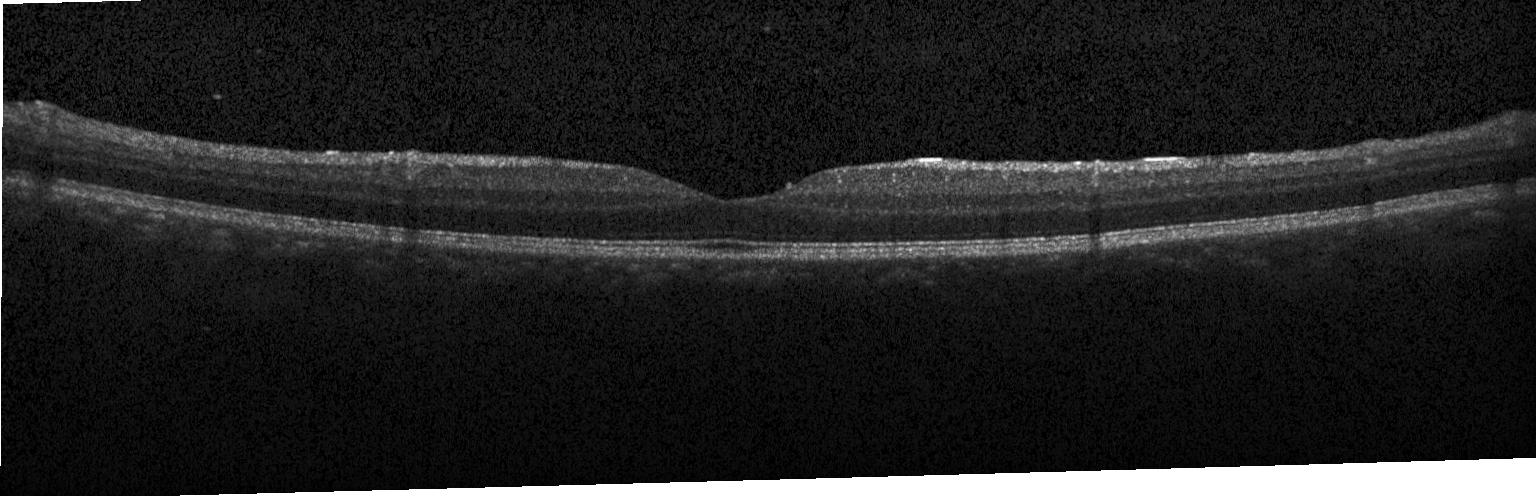 Diagnosis: no evidence of CNV, DME, or drusen.